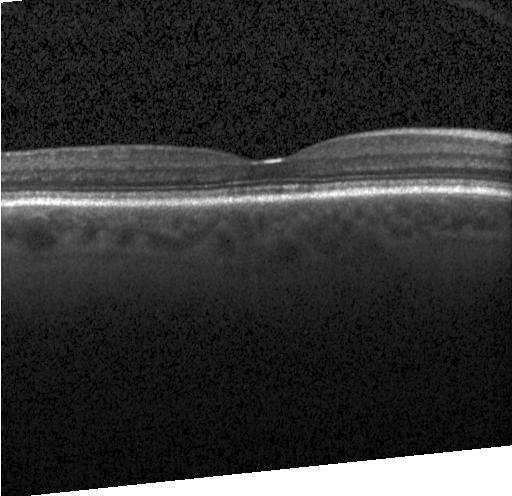

Spectral-domain optical coherence tomography; OCT B-scan. Assessment: no CNV, DME, or drusen.